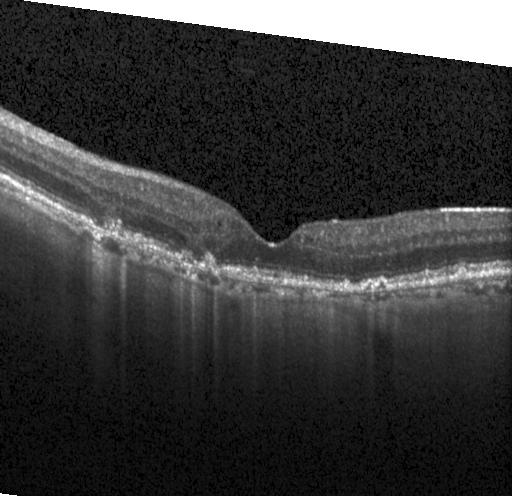
Spectral-domain optical coherence tomography · Heidelberg Spectralis · fovea-centered · retinal OCT B-scan
Diagnosis: choroidal neovascularization.